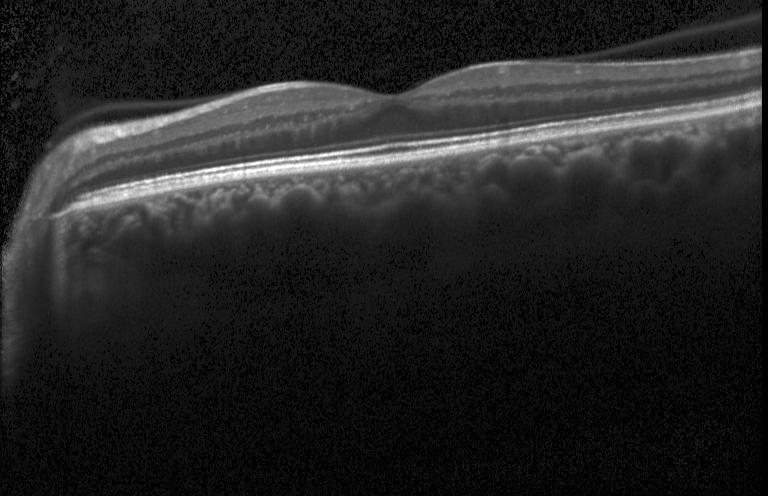

Impression: no evidence of choroidal neovascularization, diabetic macular edema, or drusen.